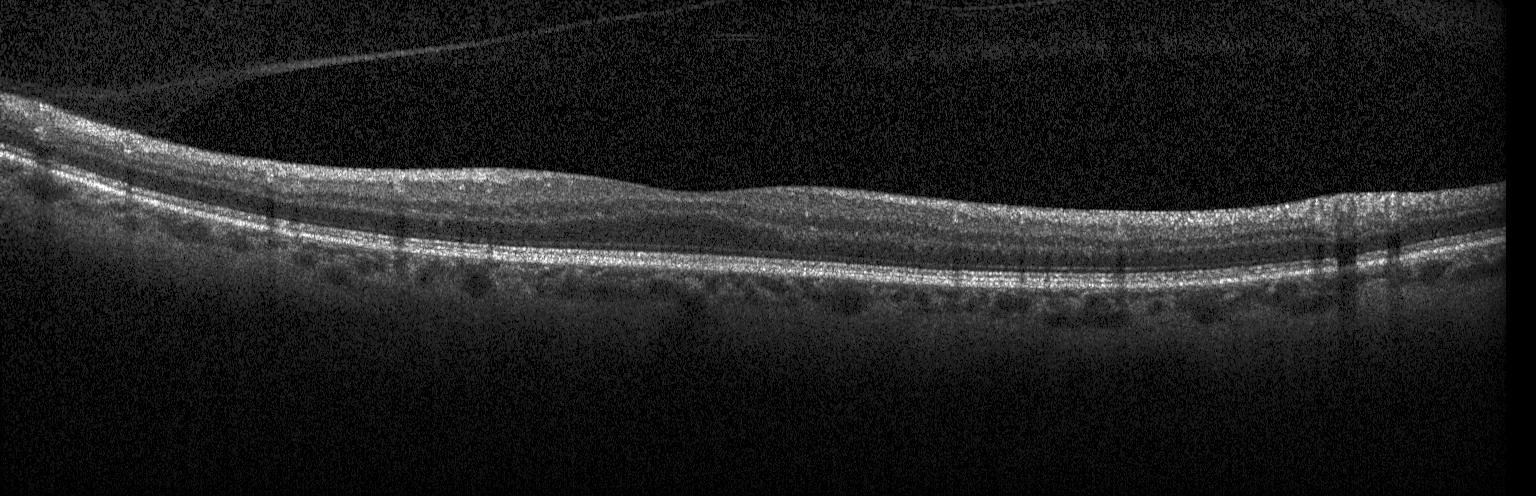 Optical coherence tomography scan — No CNV, no DME, and no drusen.